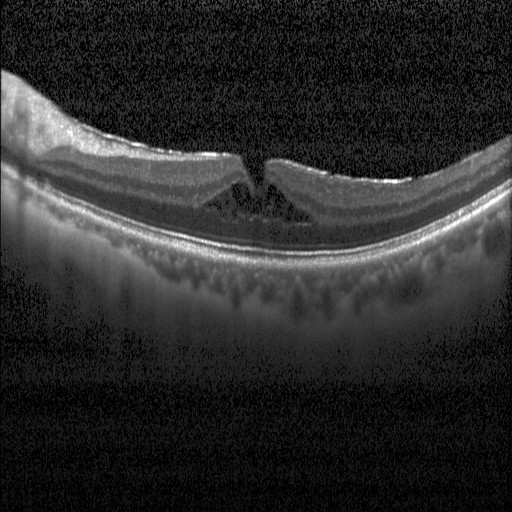

Heidelberg Spectralis; optical coherence tomography scan; spectral-domain optical coherence tomography; centered on the fovea. Assessment: DME.